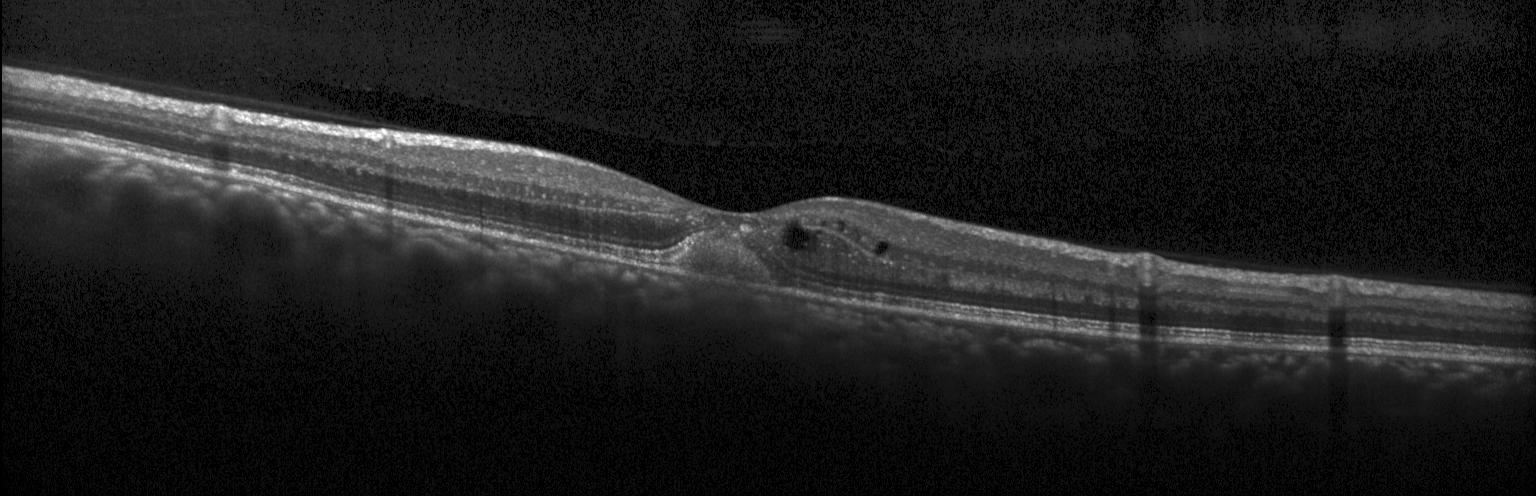

Optical coherence tomography B-scan
Dx: choroidal neovascularization.